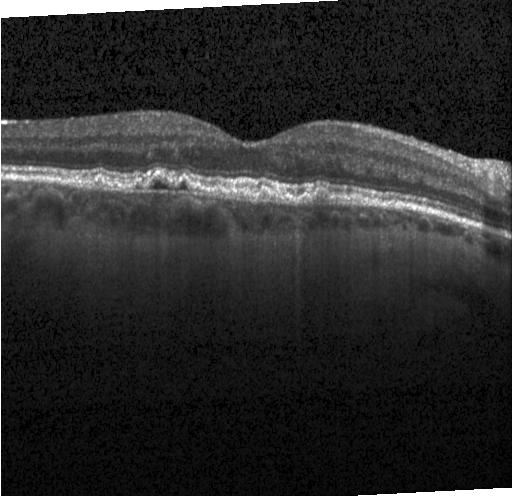

Retinal OCT B-scan, SD-OCT, horizontal scan through the fovea
Assessment: multiple drusen.